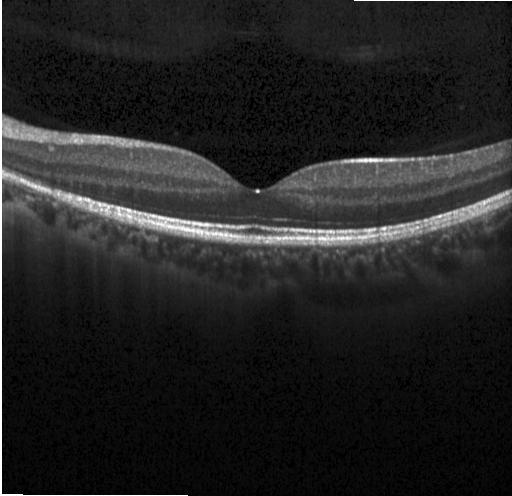
Retinal OCT B-scan · SD-OCT · Heidelberg Spectralis OCT system — The scan shows no evidence of choroidal neovascularization, diabetic macular edema, or drusen.